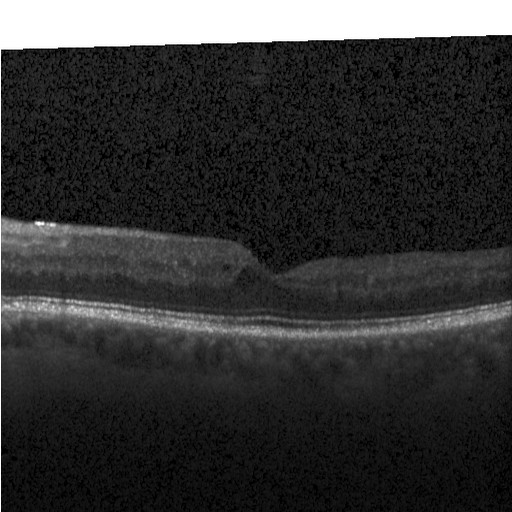

Macular OCT demonstrating diabetic macular edema.